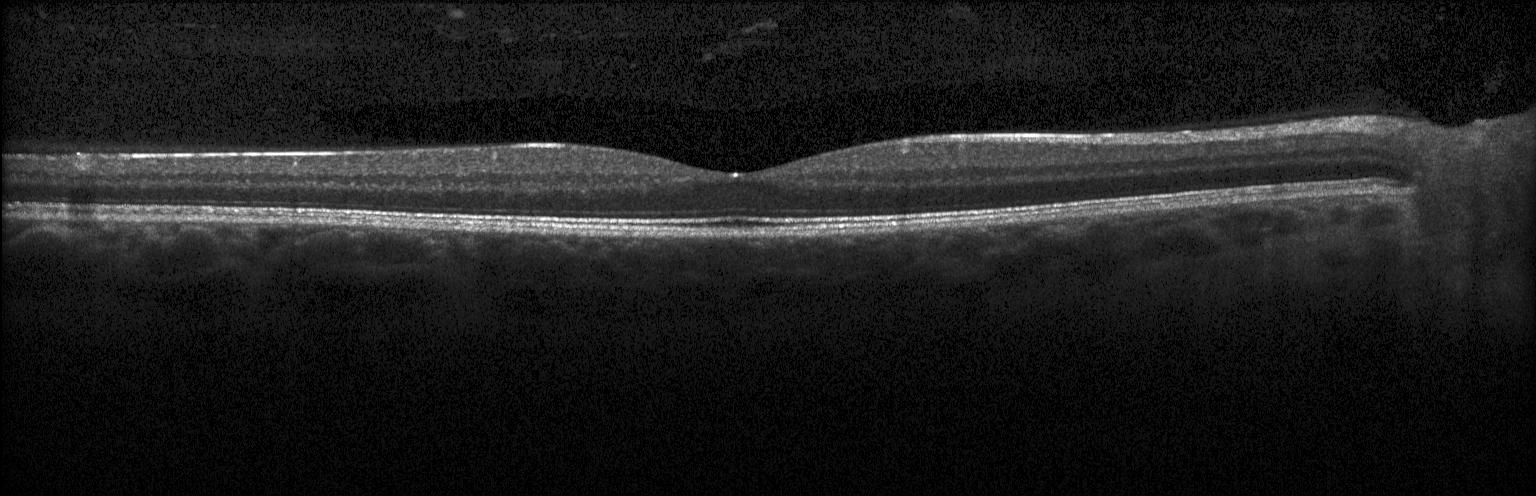 Horizontal scan through the fovea, instrument: Heidelberg Spectralis, retinal OCT cross-section.
Impression: no choroidal neovascularization, diabetic macular edema, or drusen.